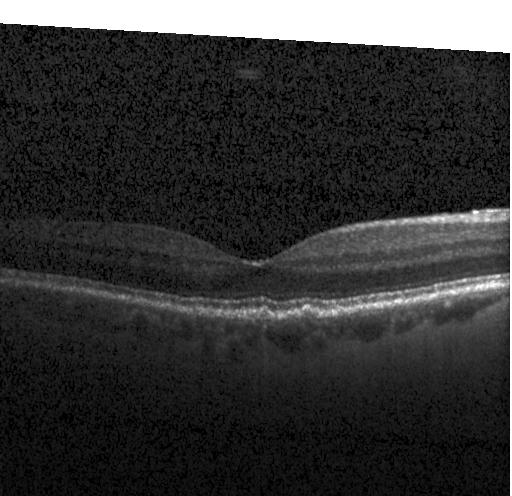

The scan shows drusen.